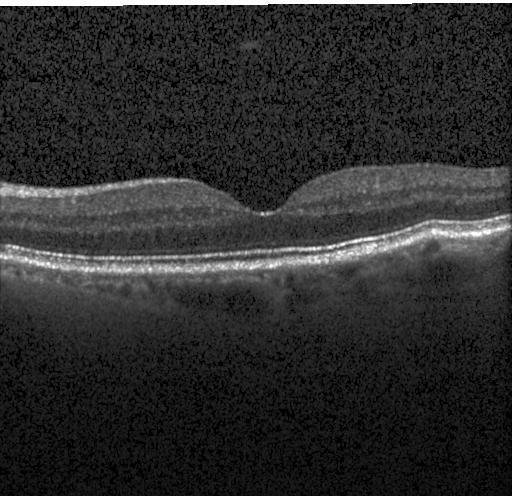 Optical coherence tomography scan. Through the macula — Finding: neither choroidal neovascularization, diabetic macular edema, nor drusen.